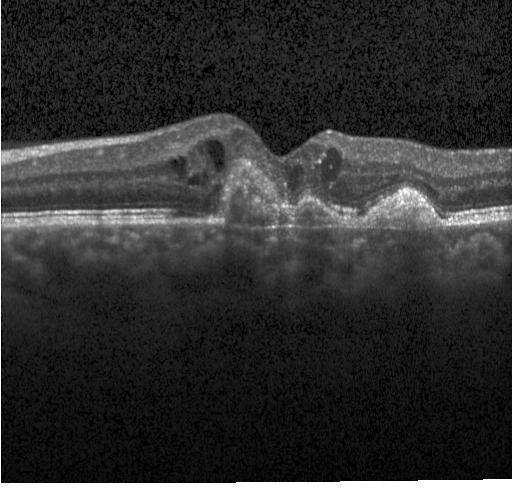 Centered on the fovea; retinal OCT cross-section
The scan shows CNV.